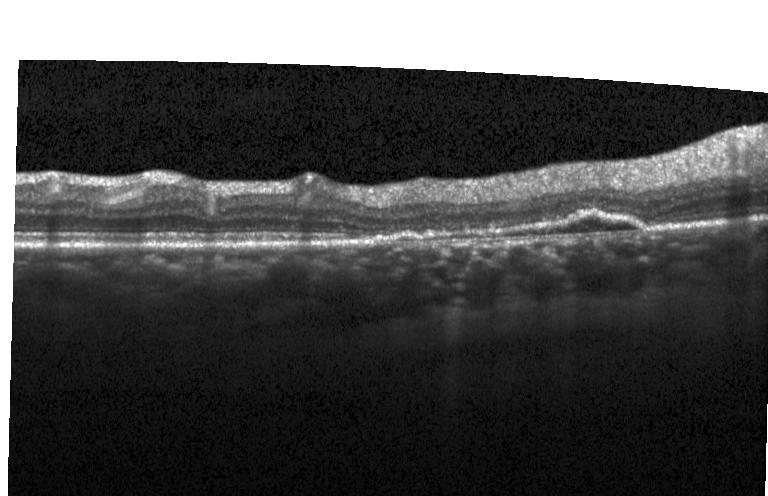

Impression: a choroidal neovascular membrane.